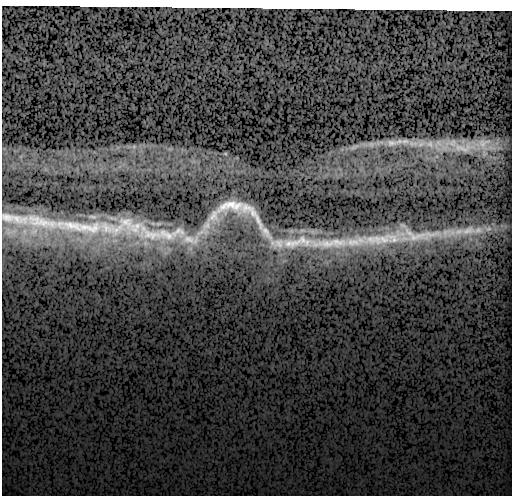 Optical coherence tomography B-scan. Fovea-centered. Spectral-domain OCT. Heidelberg Spectralis OCT system
Impression: multiple drusen.